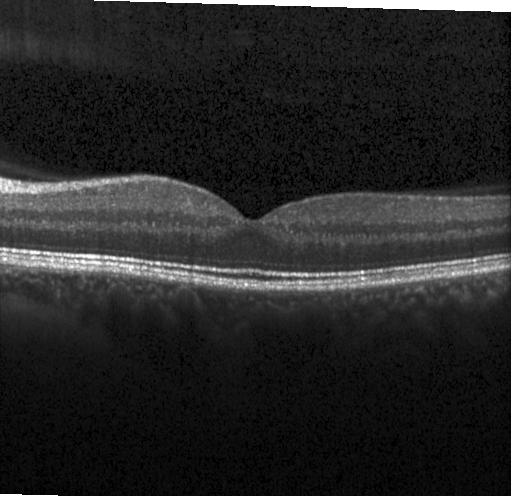
Fovea-centered, SD-OCT, optical coherence tomography B-scan
Dx: no evidence of CNV, DME, or drusen.